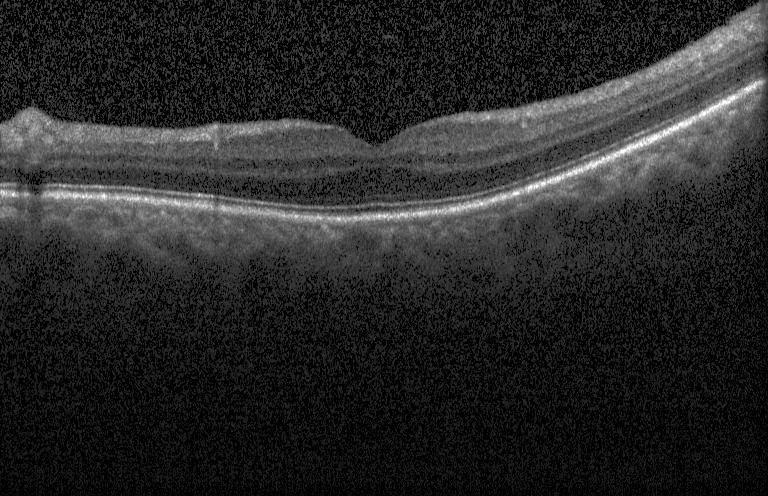
OCT B-scan showing no evidence of CNV, DME, or drusen.